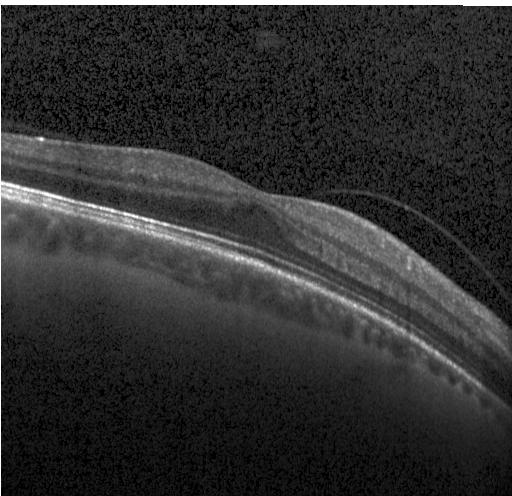
Optical coherence tomography scan — The scan shows no evidence of choroidal neovascularization, diabetic macular edema, or drusen.